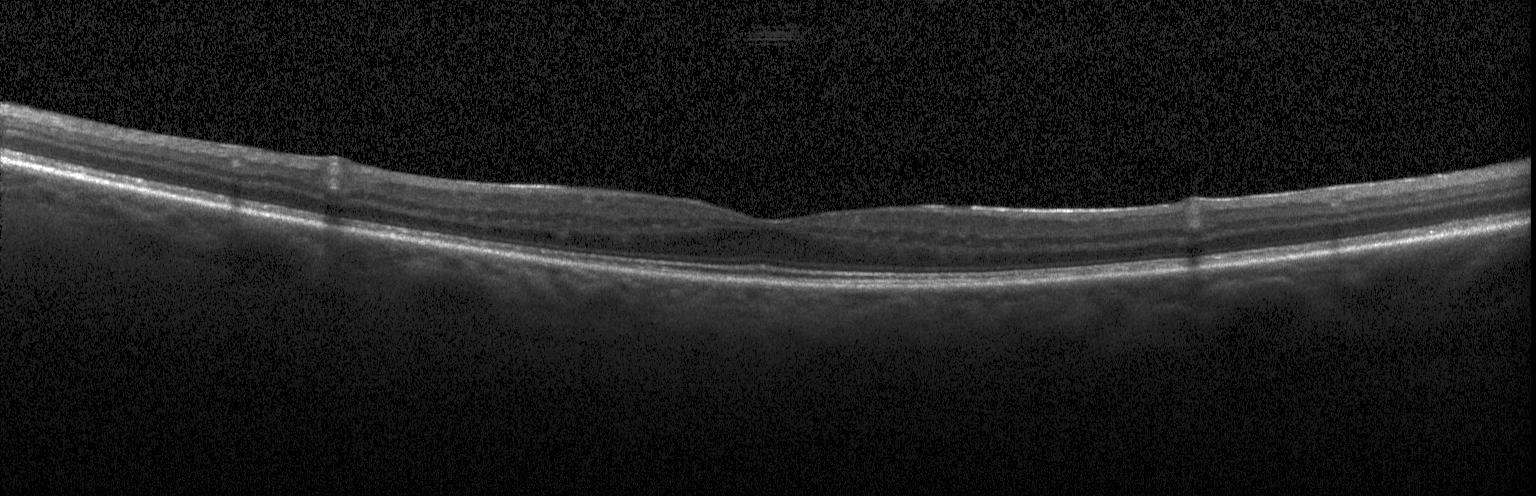 Instrument: Heidelberg Spectralis · SD-OCT · centered on the fovea · optical coherence tomography scan
Diagnosis: no choroidal neovascularization, no diabetic macular edema, and no drusen.